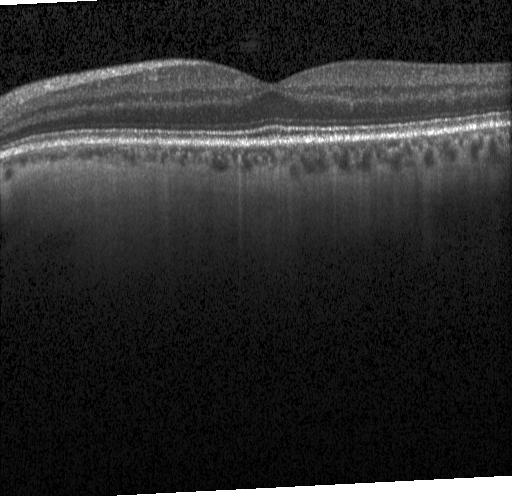

Fovea-centered · retinal OCT cross-section. Impression: no choroidal neovascularization, diabetic macular edema, or drusen.